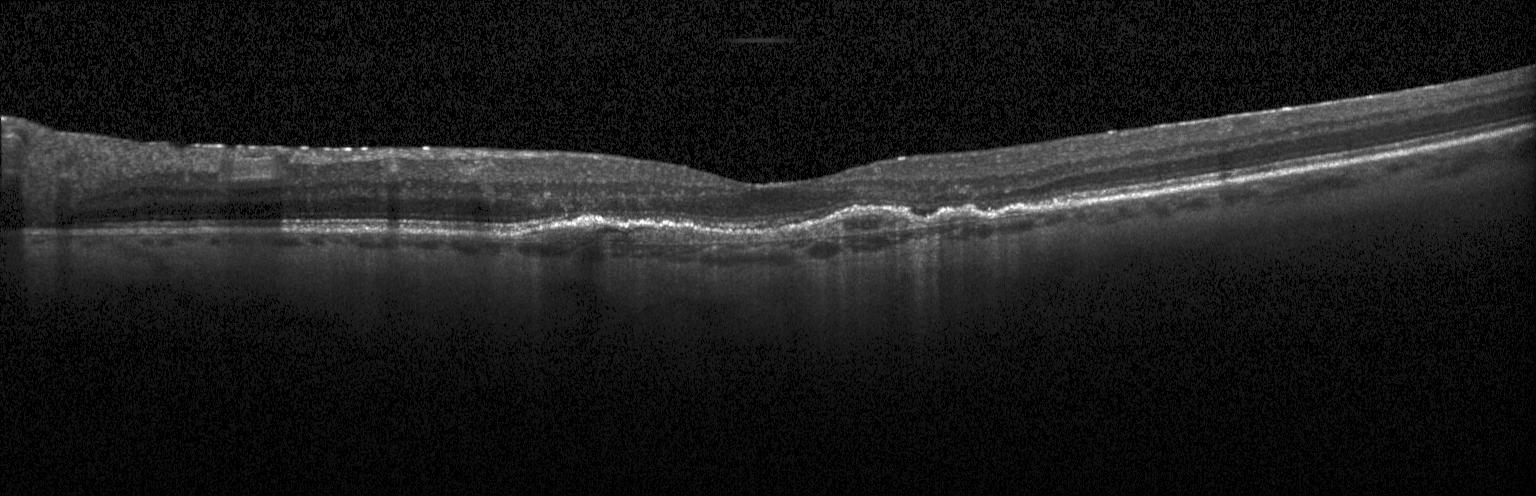 Spectral-domain optical coherence tomography, optical coherence tomography B-scan — Diagnosis: choroidal neovascularization (CNV).